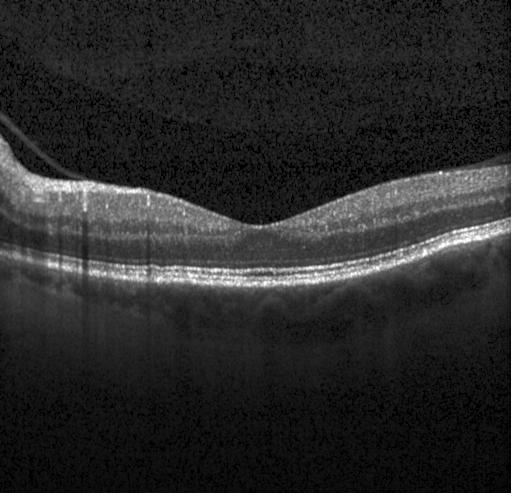
Optical coherence tomography scan. Centered on the fovea — This B-scan demonstrates no choroidal neovascularization, diabetic macular edema, or drusen.